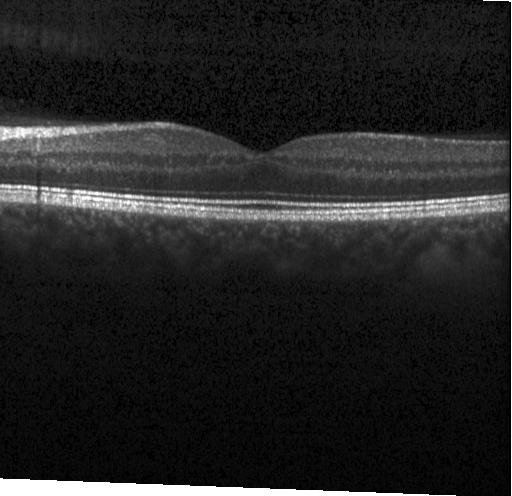 Macular OCT: no choroidal neovascularization, no diabetic macular edema, and no drusen.